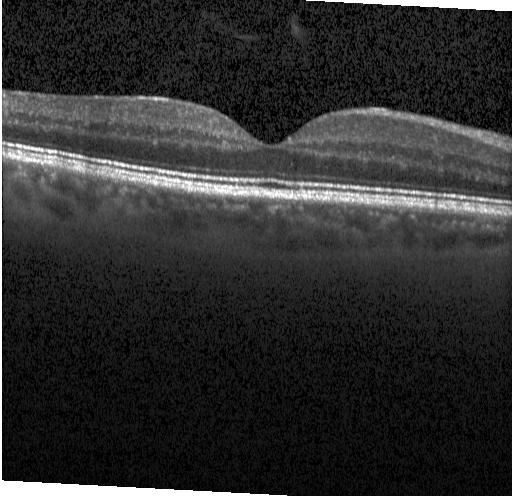
Retinal OCT B-scan — Assessment: neither choroidal neovascularization, diabetic macular edema, nor drusen.